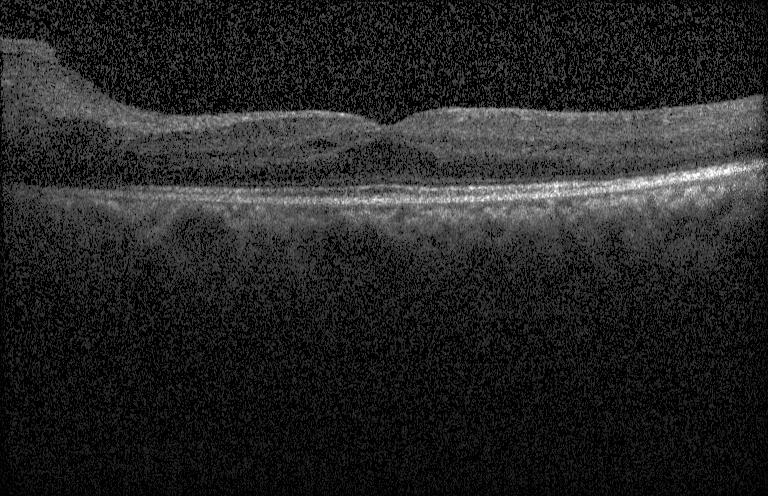

This B-scan demonstrates DME.